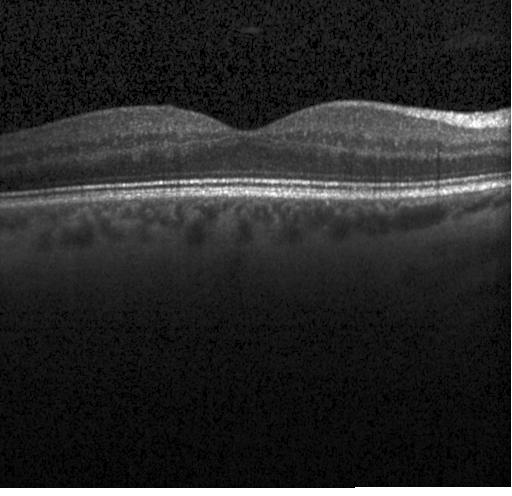 Retinal OCT cross-section
The scan shows no evidence of choroidal neovascularization, diabetic macular edema, or drusen.